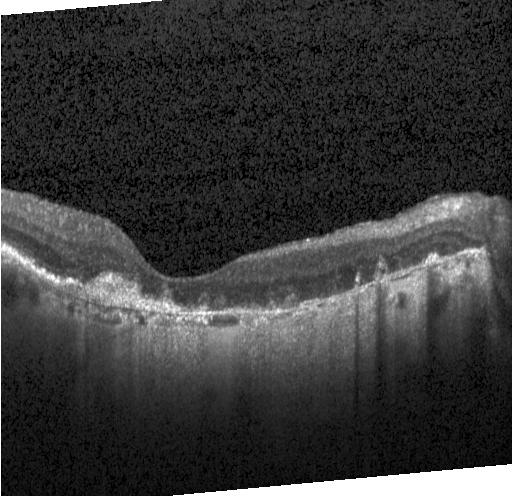
The scan shows choroidal neovascularization (CNV).